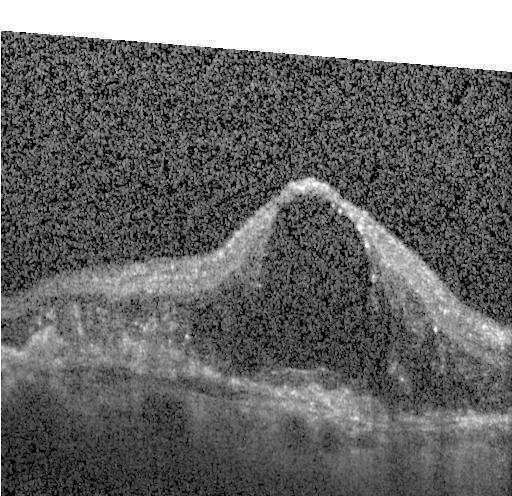
Retinal OCT cross-section. Spectral-domain OCT.
Diagnosis: a choroidal neovascular membrane.